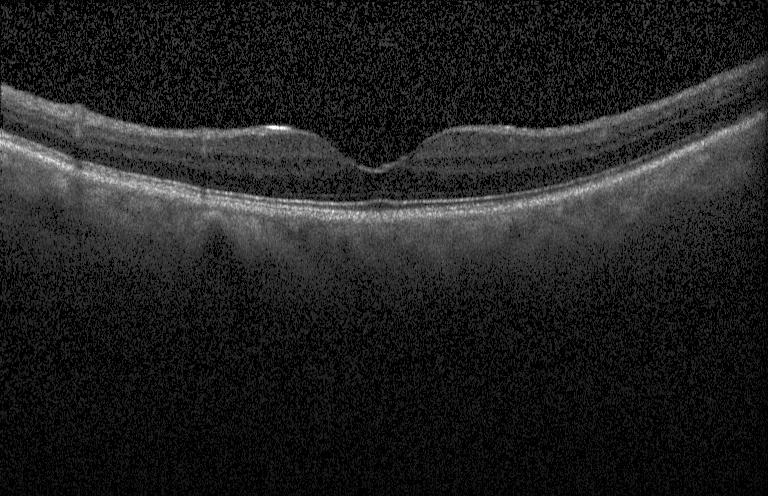

OCT B-scan. Assessment: no evidence of CNV, DME, or drusen.